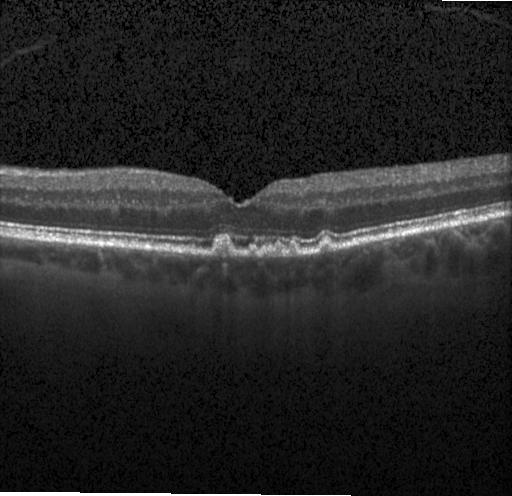
OCT B-scan — Diagnosis: sub-RPE drusenoid deposits.